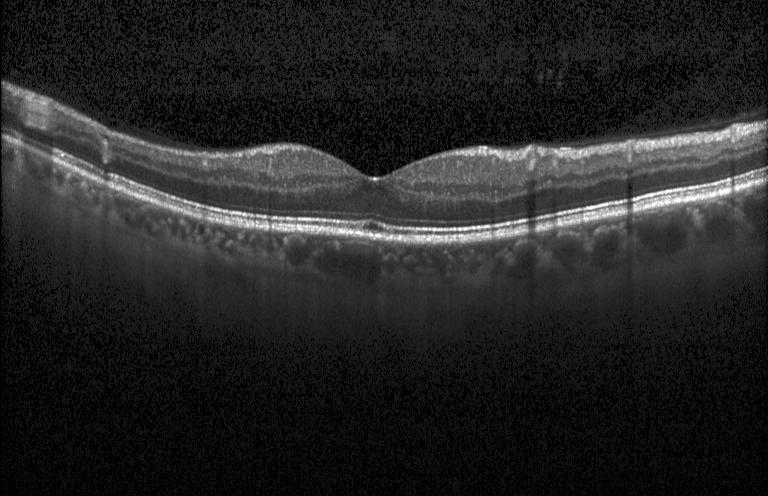
OCT line scan; macular scan; Heidelberg Spectralis.
OCT finding: no choroidal neovascularization, diabetic macular edema, or drusen.